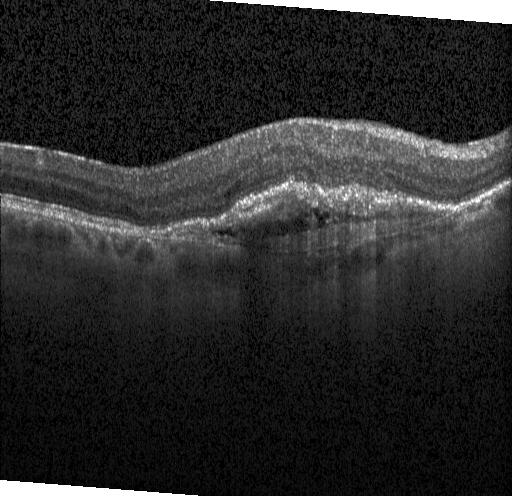 Diagnosis: a choroidal neovascular membrane.